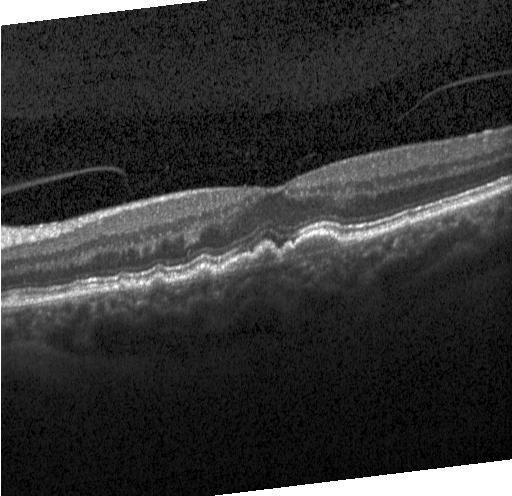 Finding: choroidal neovascularization.